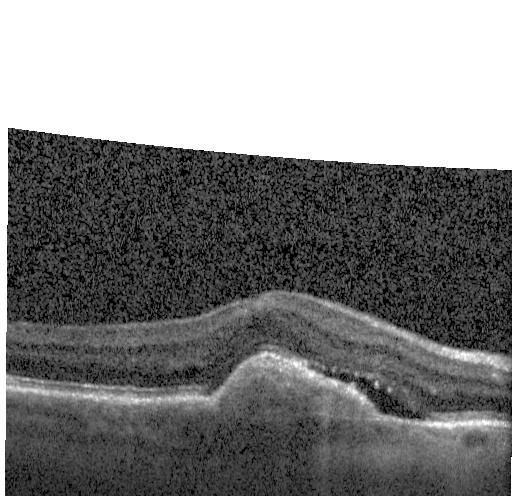 Retinal OCT cross-section
Diagnosis: choroidal neovascularization.